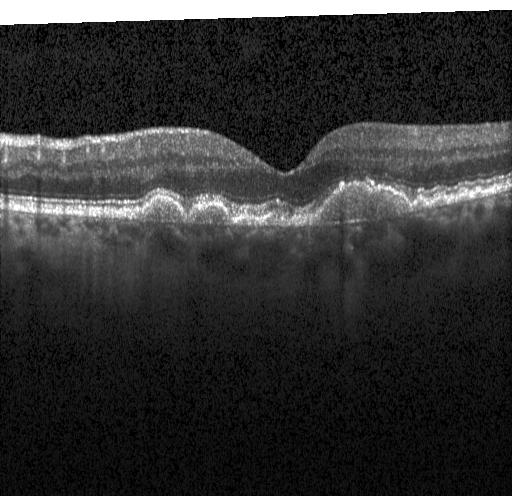

Retinal OCT B-scan · acquired on a Heidelberg Spectralis
Impression: multiple drusen.